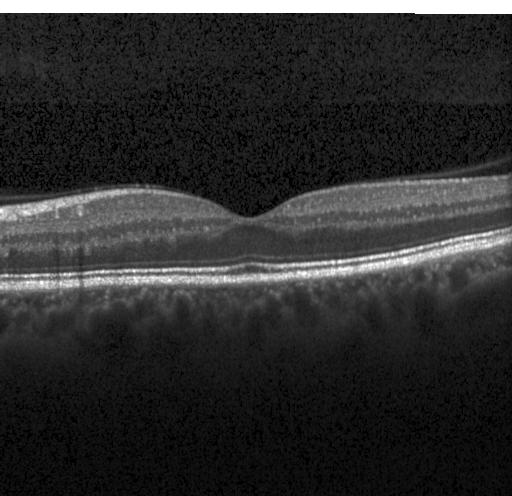

Retinal OCT cross-section showing neither choroidal neovascularization, diabetic macular edema, nor drusen.